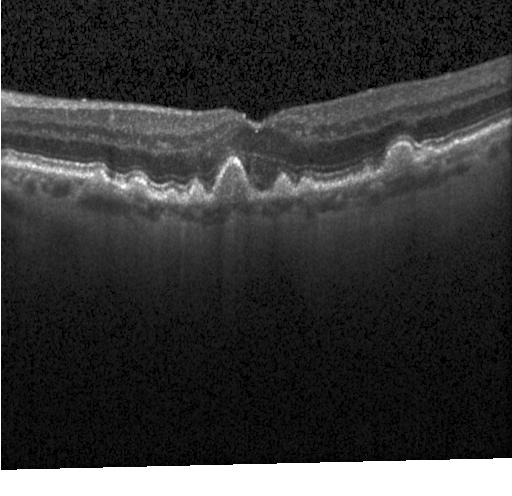 OCT finding: multiple drusen.